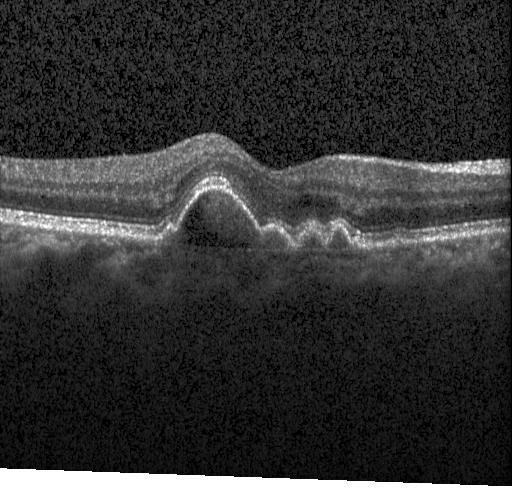
Finding: choroidal neovascularization.